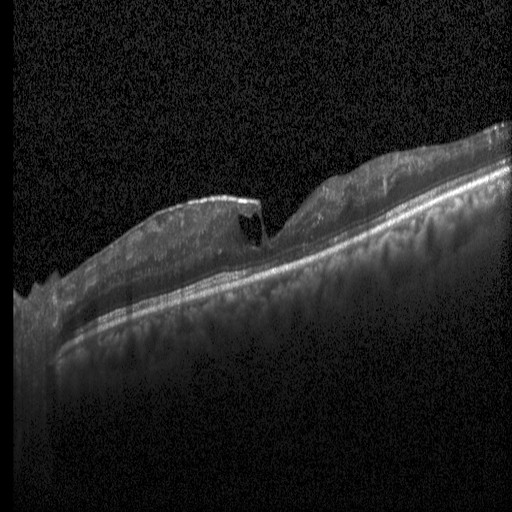

Spectral-domain optical coherence tomography, optical coherence tomography B-scan, through the macula
DME.